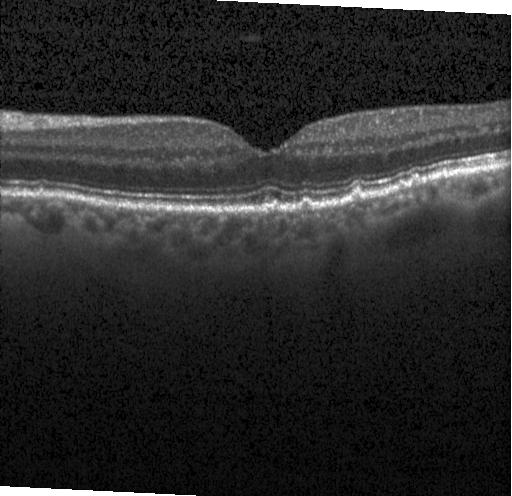 Retinal OCT B-scan — Diagnosis: drusen.